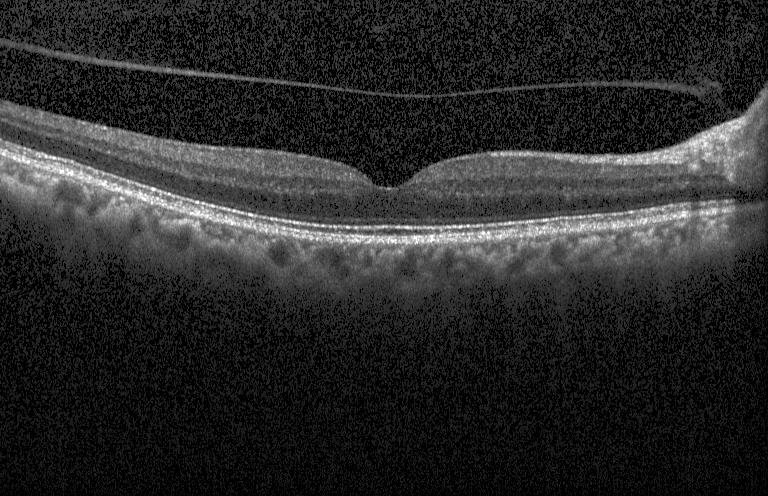 Macular OCT: neither CNV, DME, nor drusen.